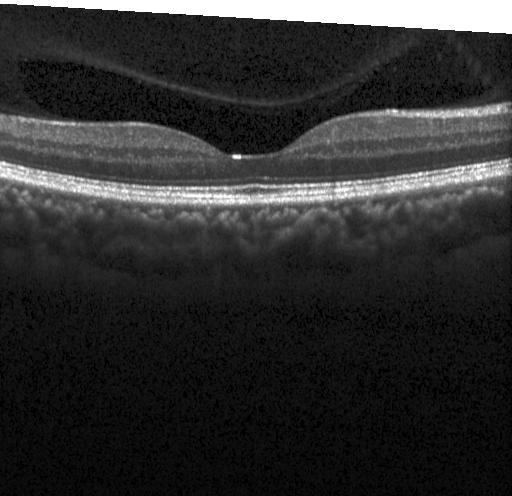 Diagnosis: neither CNV, DME, nor drusen.